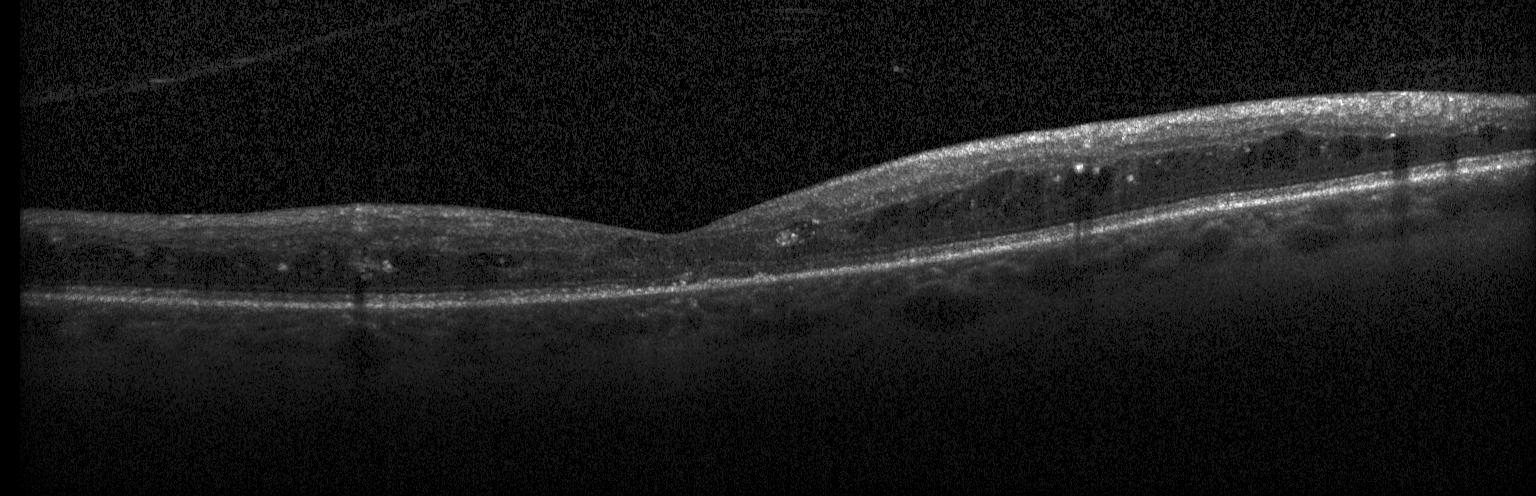
Spectral-domain OCT; macular scan; Heidelberg Spectralis; OCT line scan
Assessment: diabetic macular edema.